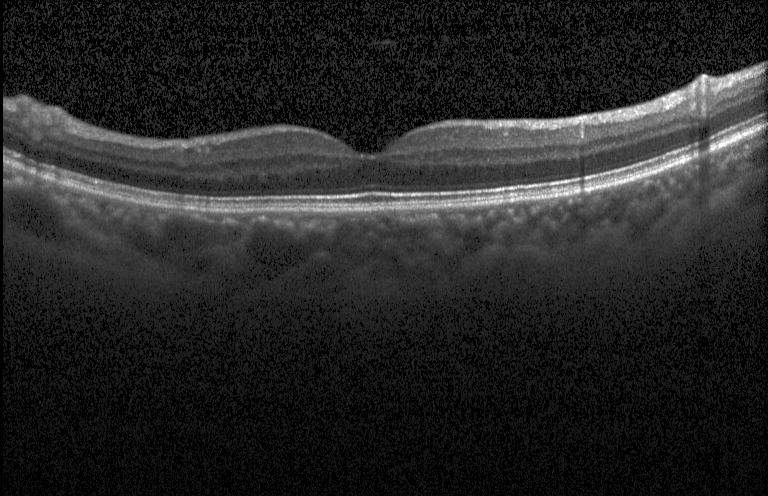 Through the macula. Spectral-domain optical coherence tomography. Optical coherence tomography scan. The scan shows neither choroidal neovascularization, diabetic macular edema, nor drusen.